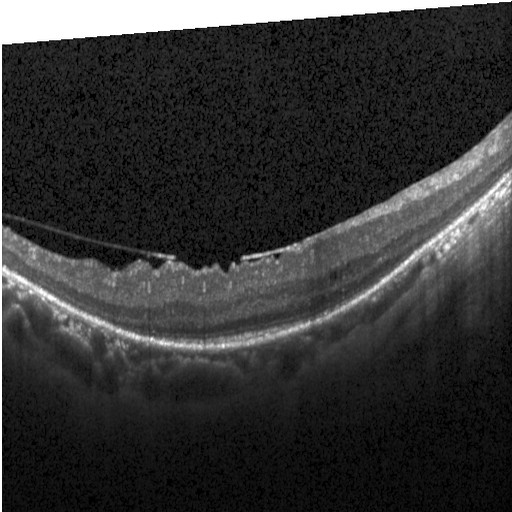

Macular OCT demonstrating diabetic macular edema (DME).